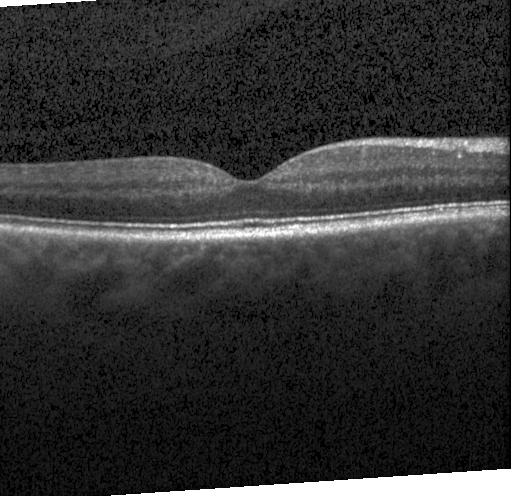

SD-OCT. Centered on the fovea. Optical coherence tomography scan.
Macular OCT: no CNV, no DME, and no drusen.